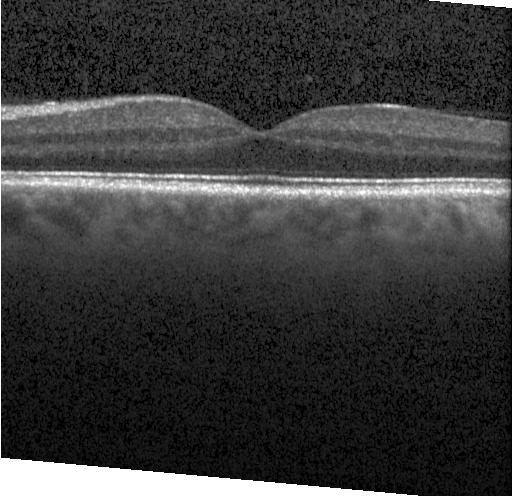 Optical coherence tomography B-scan. Fovea-centered. Heidelberg Spectralis OCT system. Impression: no evidence of choroidal neovascularization, diabetic macular edema, or drusen.